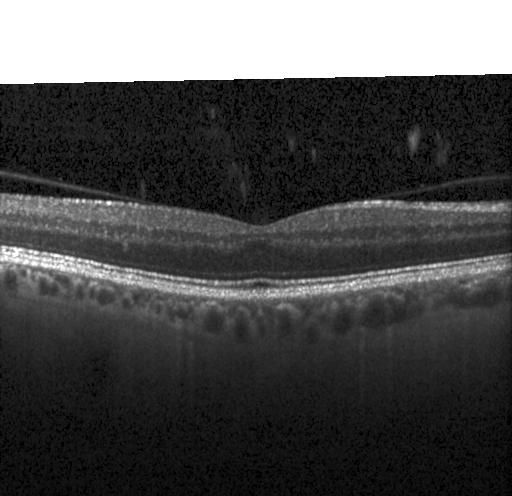
Spectral-domain optical coherence tomography, retinal OCT cross-section, centered on the fovea.
Macular OCT: no CNV, no DME, and no drusen.